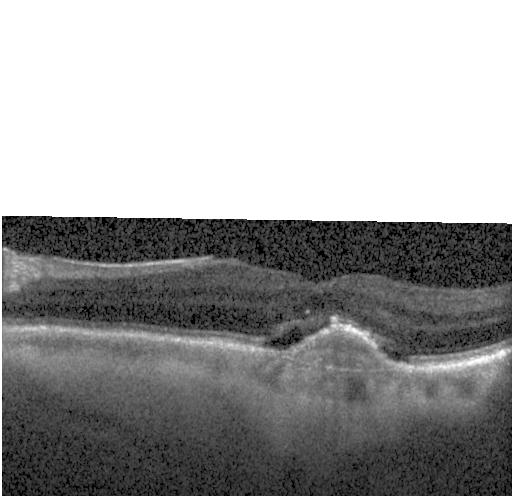
Optical coherence tomography B-scan
This B-scan demonstrates choroidal neovascularization (CNV).